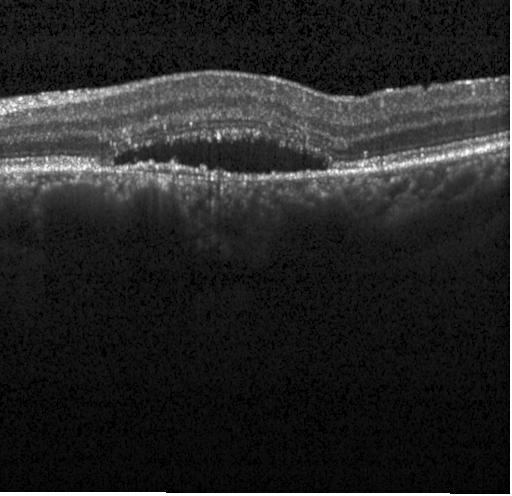 Macular OCT: choroidal neovascularization (CNV).